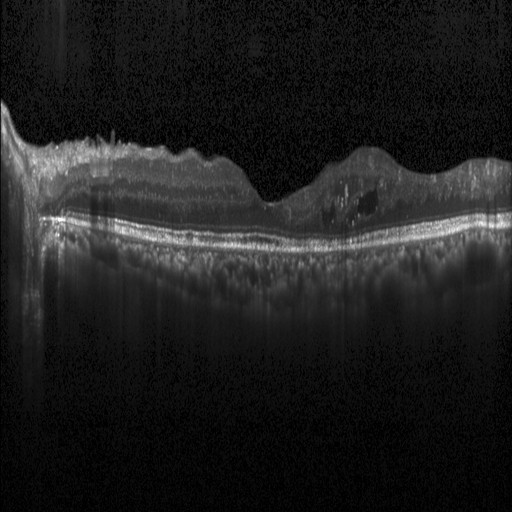
Spectral-domain optical coherence tomography · optical coherence tomography scan. Finding: DME.